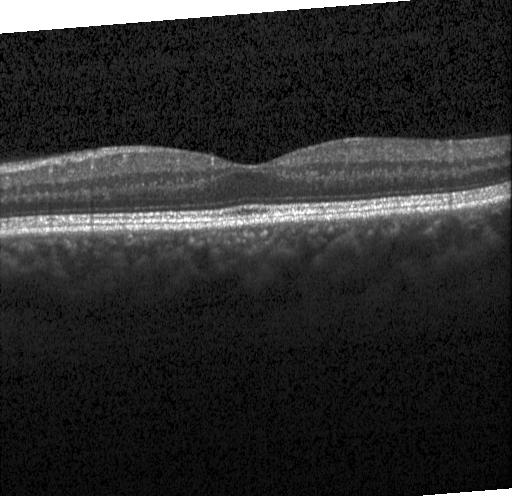 Instrument: Heidelberg Spectralis · optical coherence tomography scan
Diagnosis: no evidence of choroidal neovascularization, diabetic macular edema, or drusen.